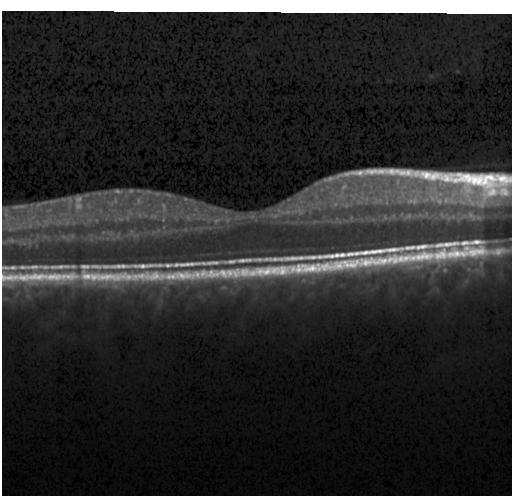

Macular OCT demonstrating no choroidal neovascularization, diabetic macular edema, or drusen.